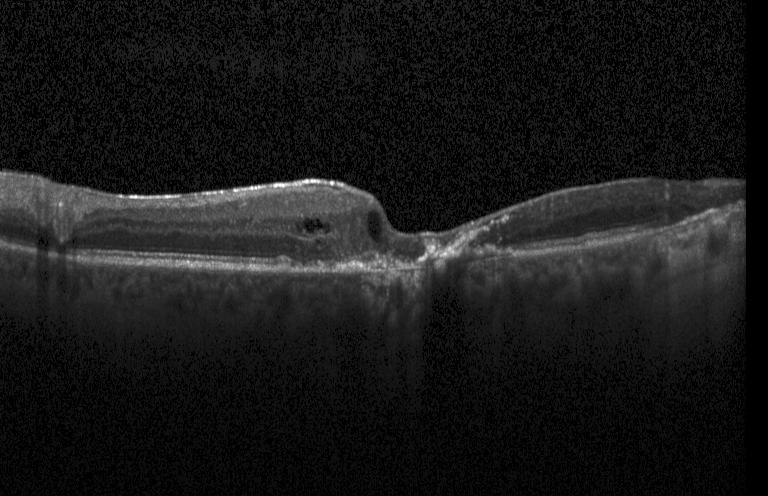

Horizontal scan through the fovea. Retinal OCT B-scan
Finding: a choroidal neovascular membrane.